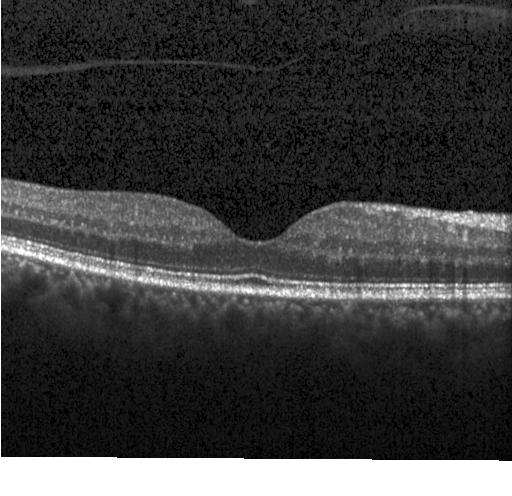 Retinal OCT cross-section. Diagnosis: no CNV, DME, or drusen.